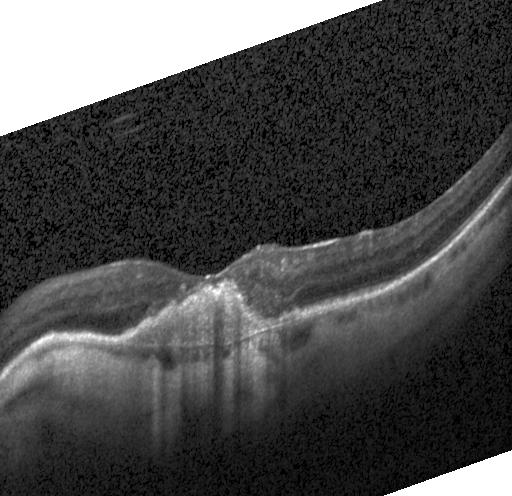 Instrument: Heidelberg Spectralis · horizontal scan through the fovea · SD-OCT · OCT line scan — Assessment: choroidal neovascularization (CNV).